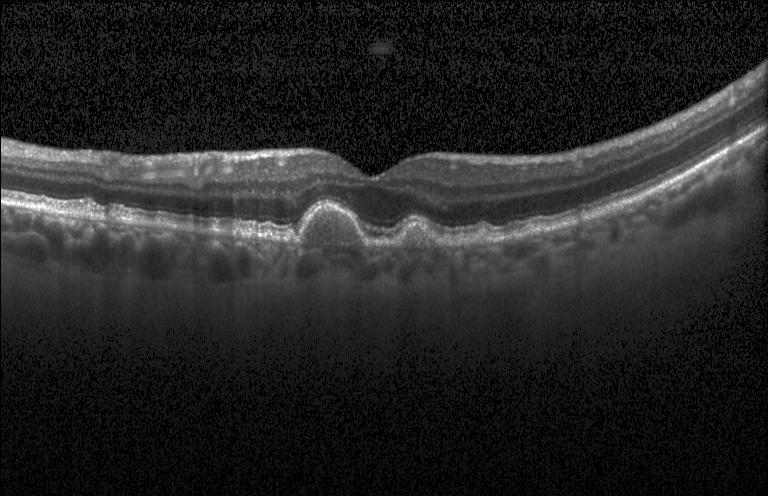
Macular OCT: multiple drusen.